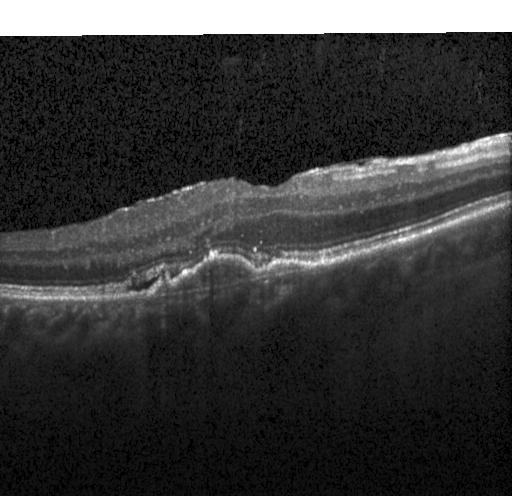
Acquired on a Heidelberg Spectralis; centered on the fovea; OCT B-scan — Macular OCT: a choroidal neovascular membrane.